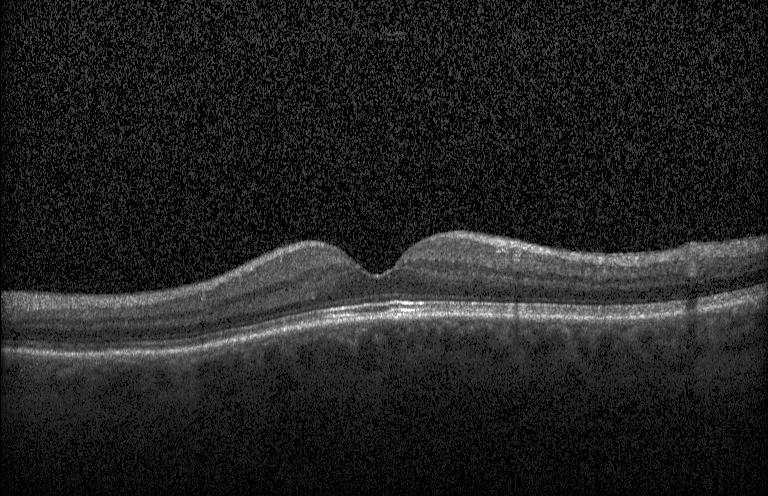

Assessment: no choroidal neovascularization, no diabetic macular edema, and no drusen.